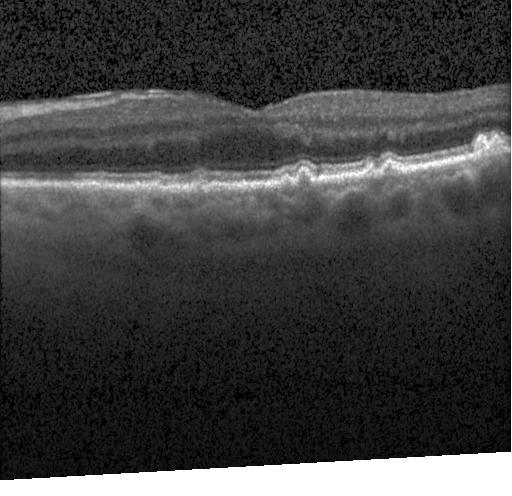

Fovea-centered; acquired on a Heidelberg Spectralis; spectral-domain optical coherence tomography; OCT B-scan
Drusen.